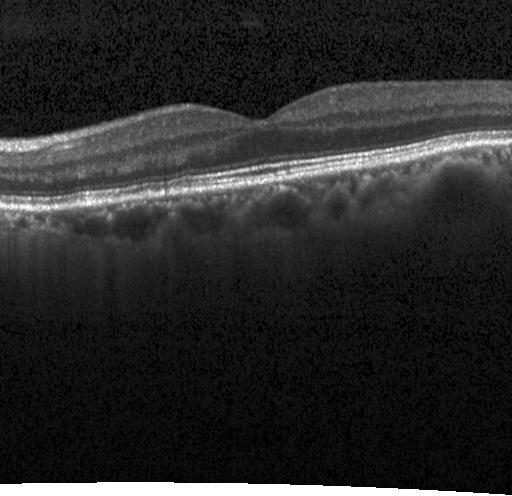 Instrument: Heidelberg Spectralis. OCT B-scan. SD-OCT. Impression: no evidence of CNV, DME, or drusen.